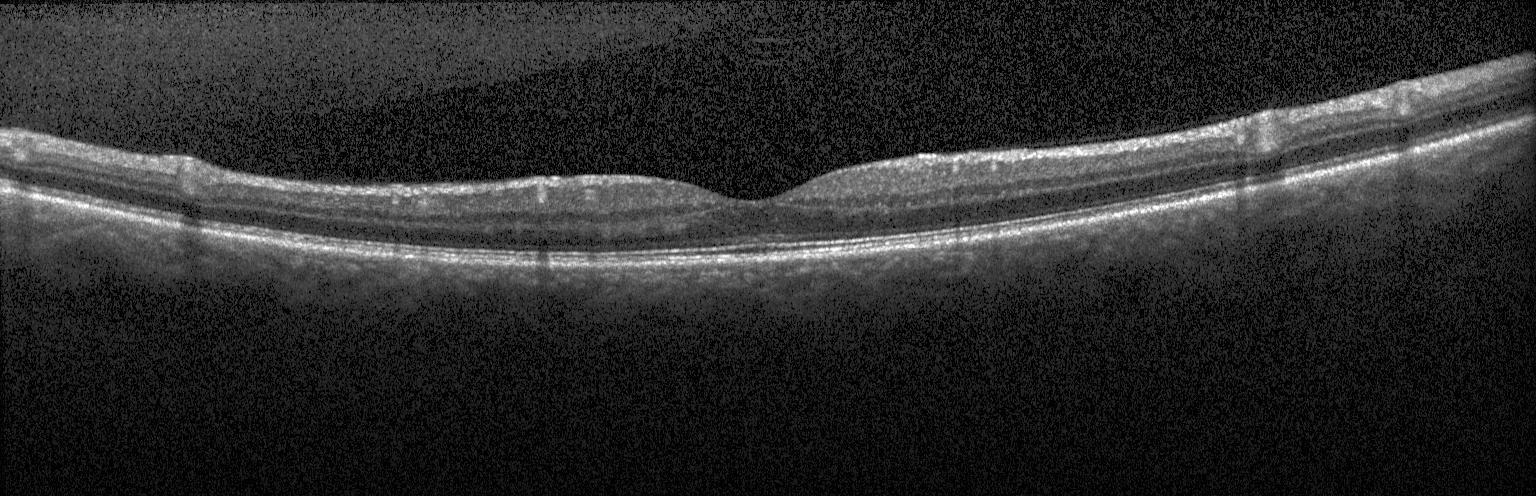 Spectral-domain OCT B-scan: no choroidal neovascularization, no diabetic macular edema, and no drusen.